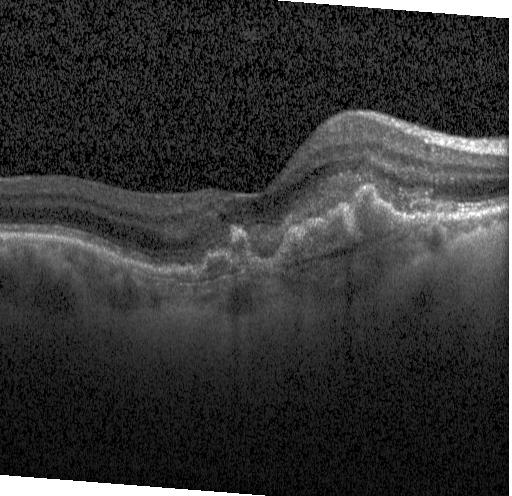 Spectral-domain OCT B-scan: CNV.